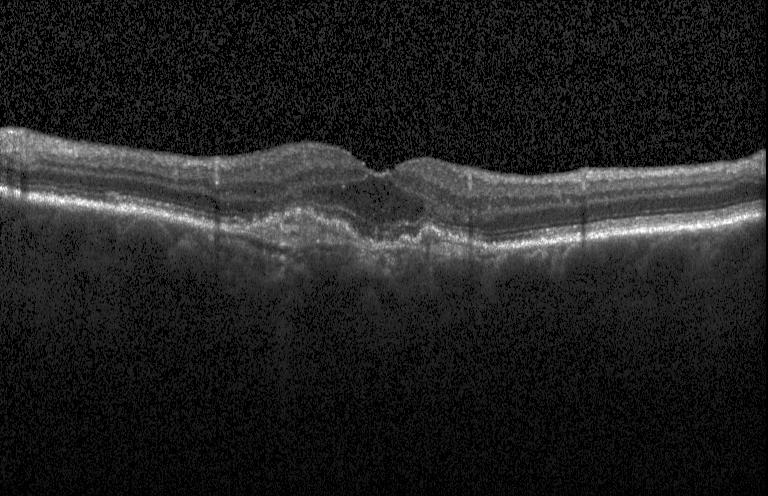

Retinal OCT B-scan
Finding: choroidal neovascularization.